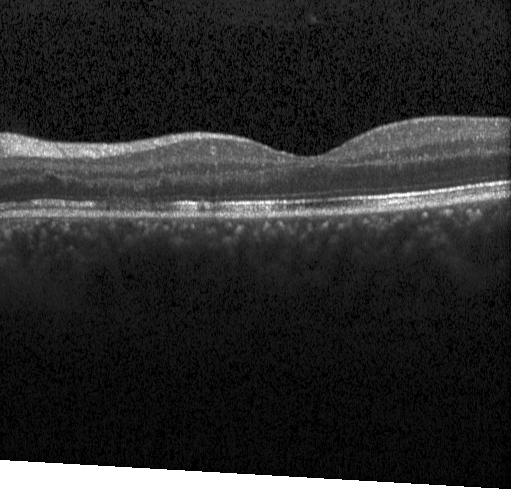
Retinal OCT B-scan, SD-OCT, horizontal scan through the fovea — Finding: neither choroidal neovascularization, diabetic macular edema, nor drusen.